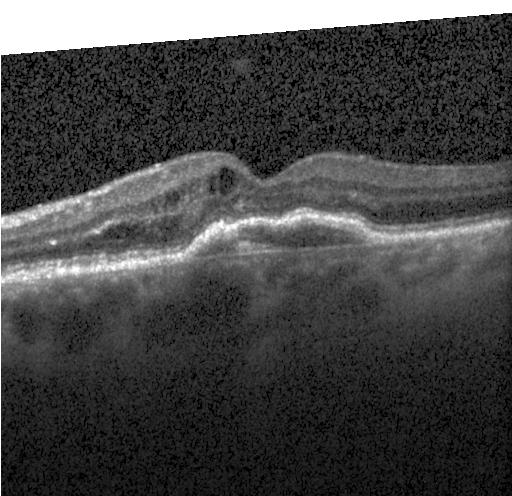

Macular OCT demonstrating CNV.